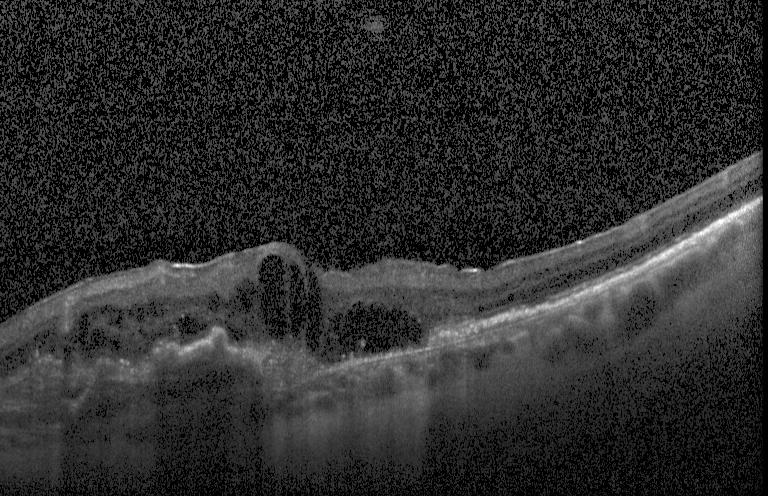 Retinal OCT B-scan. Assessment: a choroidal neovascular membrane.